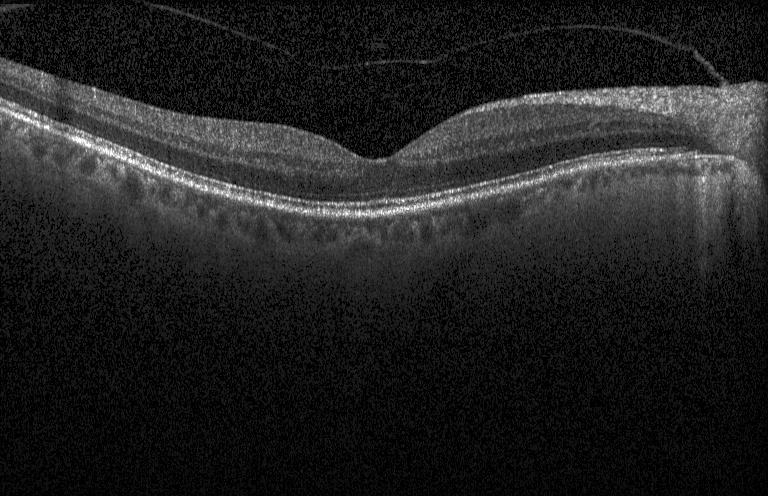 The scan shows no CNV, DME, or drusen.